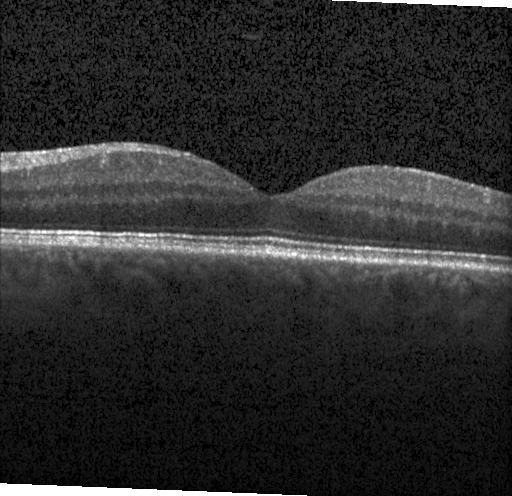 The scan shows no choroidal neovascularization, no diabetic macular edema, and no drusen.